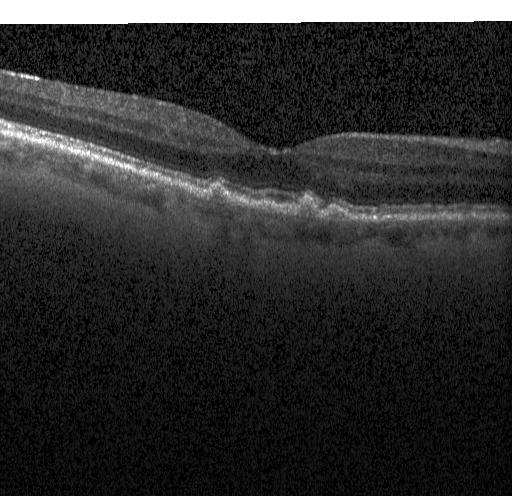

OCT B-scan. Fovea-centered. Spectral-domain OCT. Heidelberg Spectralis
Impression: drusen.